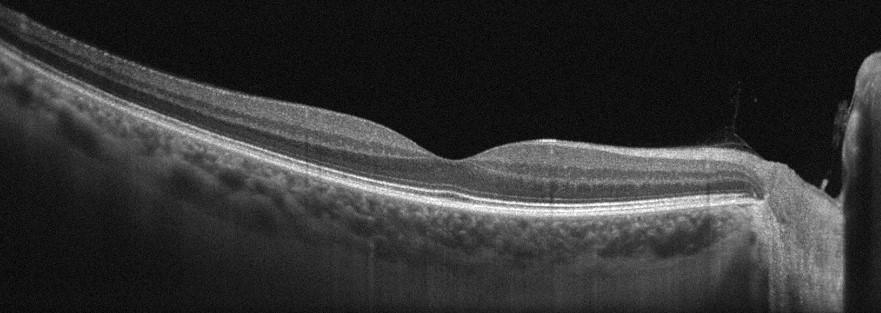 Retinal OCT B-scan, acquired on an Optovue Avanti RTVue XR, macular scan — This B-scan demonstrates no AMD, DME, ERM, RAO, RVO, or VID.